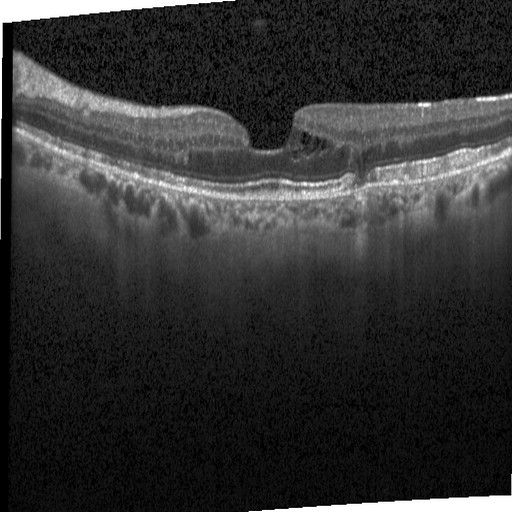
This B-scan demonstrates diabetic macular edema (DME).